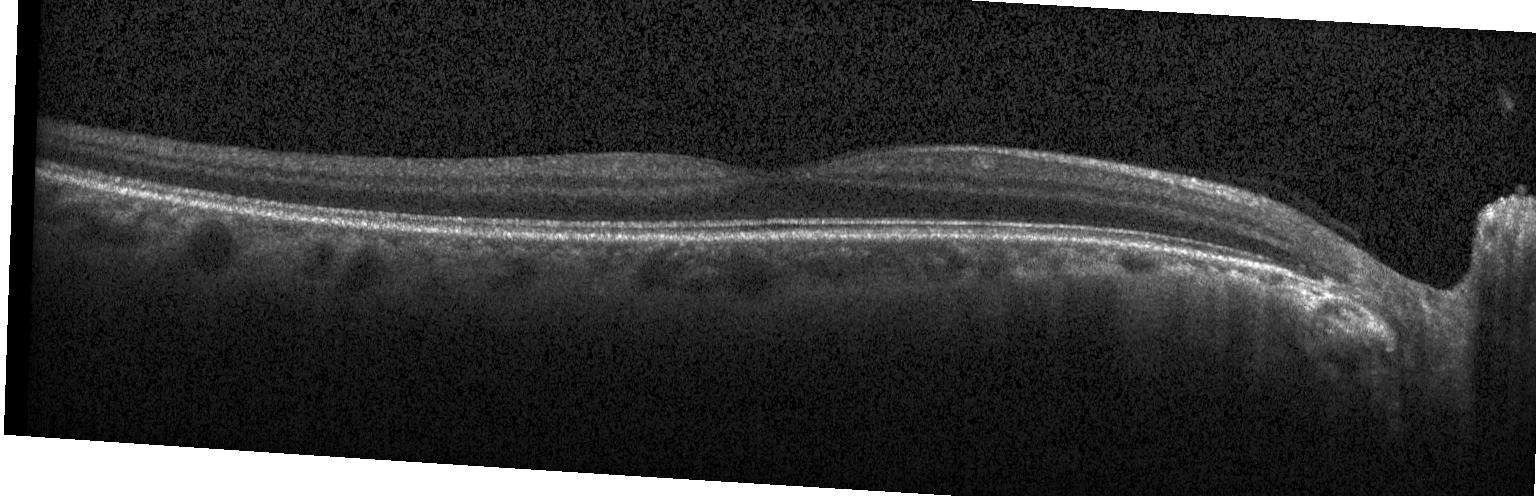

Macular OCT demonstrating no choroidal neovascularization, diabetic macular edema, or drusen.